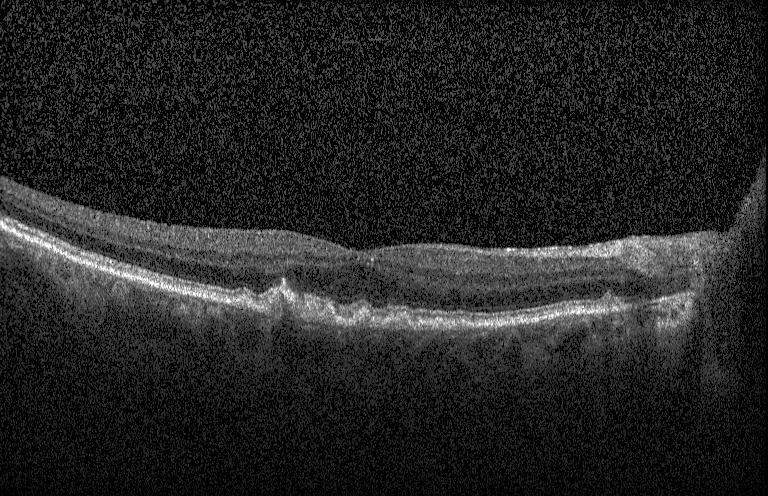 Dx: sub-RPE drusenoid deposits.